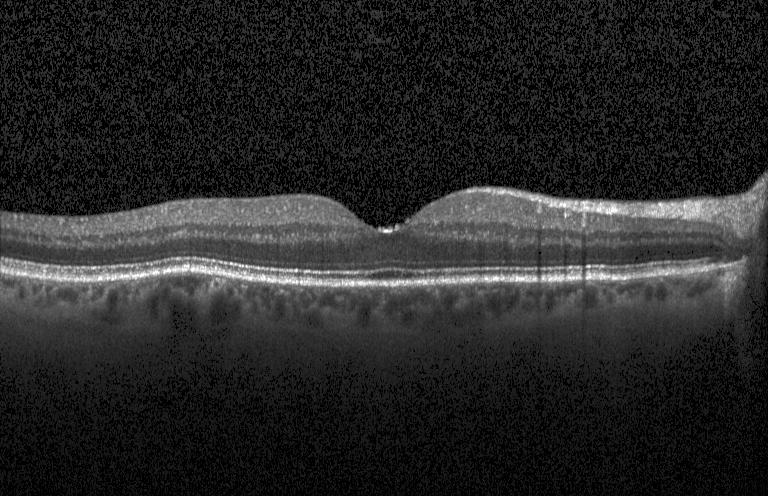

Heidelberg Spectralis OCT system. SD-OCT. Retinal OCT cross-section. Macular scan. Finding: neither choroidal neovascularization, diabetic macular edema, nor drusen.